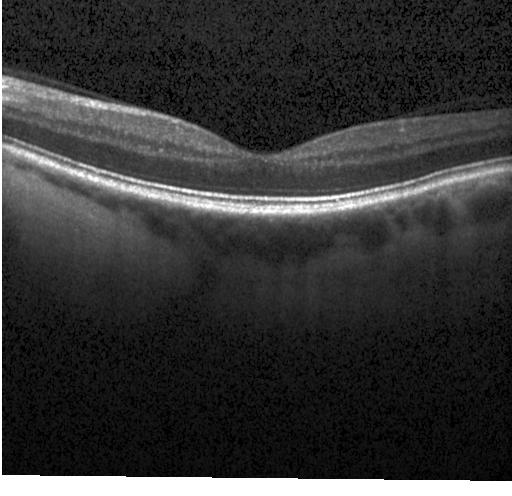
Assessment: no CNV, no DME, and no drusen.